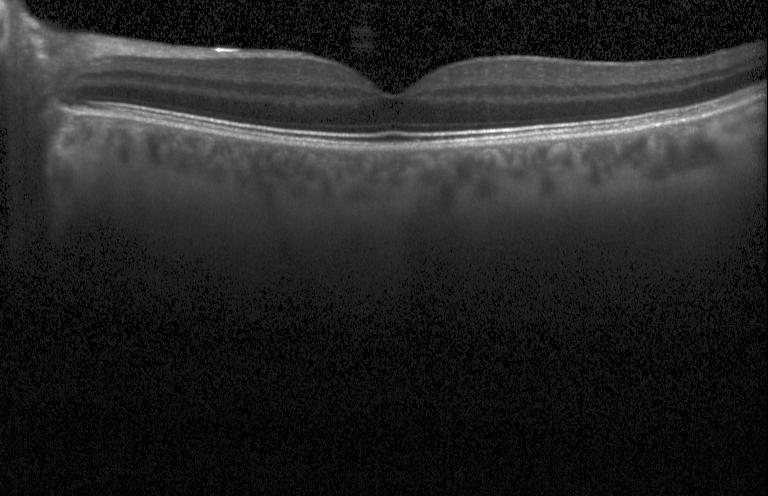 OCT line scan, spectral-domain OCT.
Impression: neither CNV, DME, nor drusen.